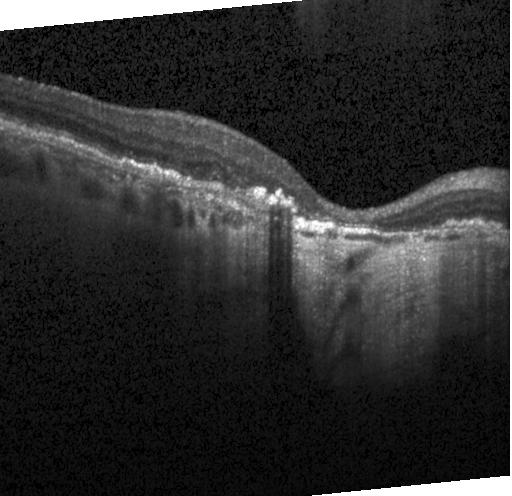
Heidelberg Spectralis, optical coherence tomography B-scan — Dx: choroidal neovascularization.